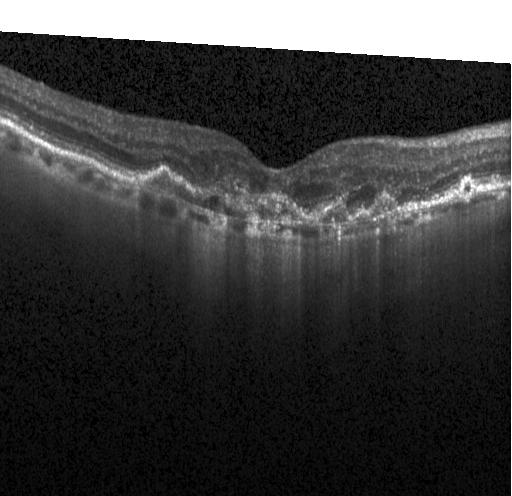
Instrument: Heidelberg Spectralis, SD-OCT, retinal OCT cross-section.
Impression: a choroidal neovascular membrane.